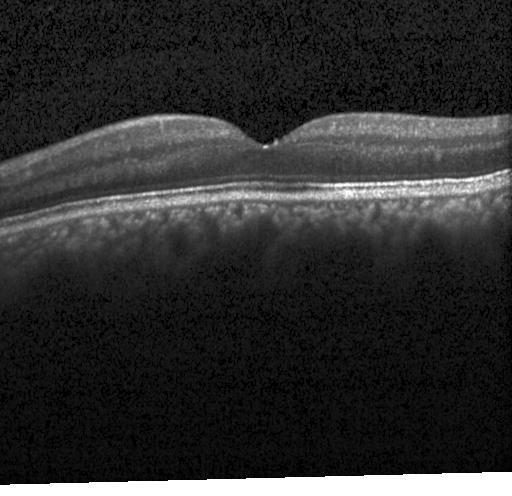 Finding: no choroidal neovascularization, no diabetic macular edema, and no drusen.